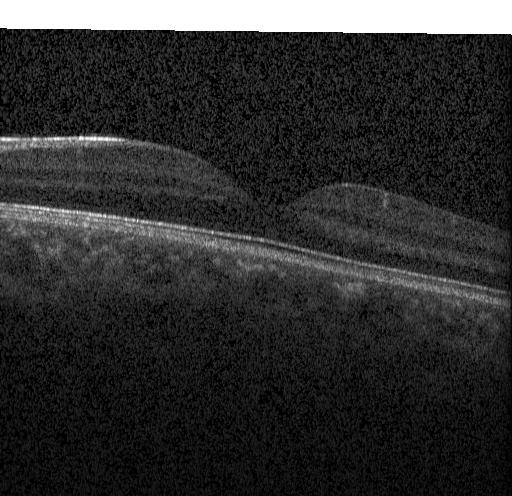 Optical coherence tomography B-scan; instrument: Heidelberg Spectralis.
Diagnosis: no evidence of CNV, DME, or drusen.